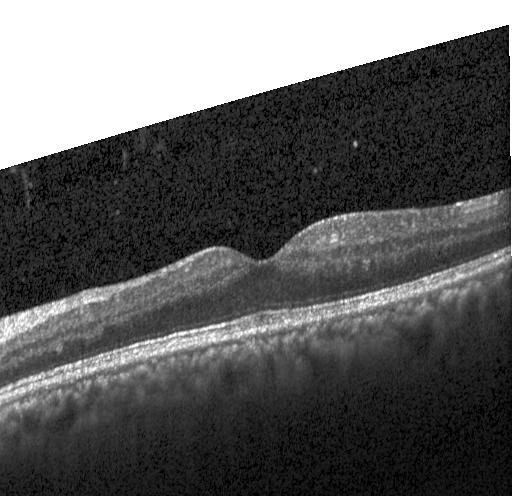

Retinal OCT cross-section showing neither choroidal neovascularization, diabetic macular edema, nor drusen.